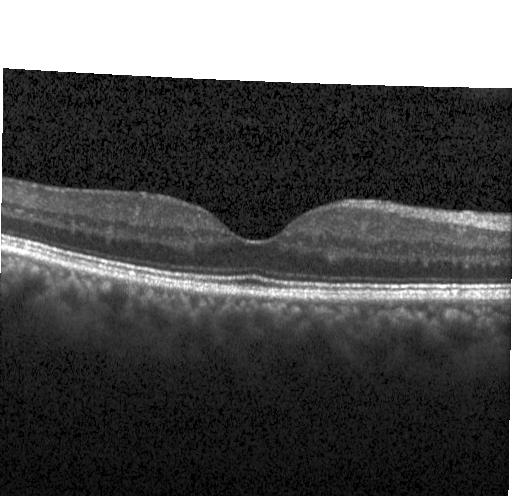

Optical coherence tomography scan. The scan shows no choroidal neovascularization, no diabetic macular edema, and no drusen.